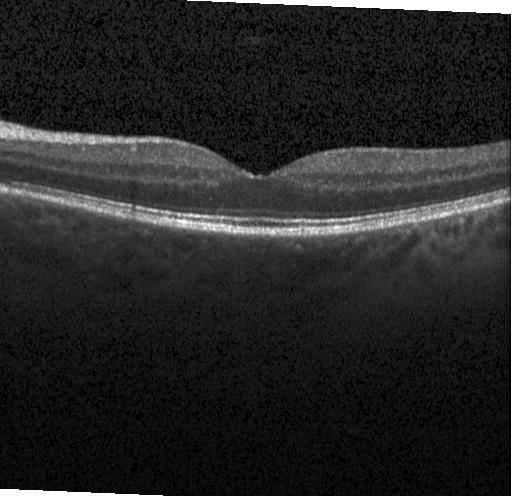 Finding: no choroidal neovascularization, no diabetic macular edema, and no drusen.